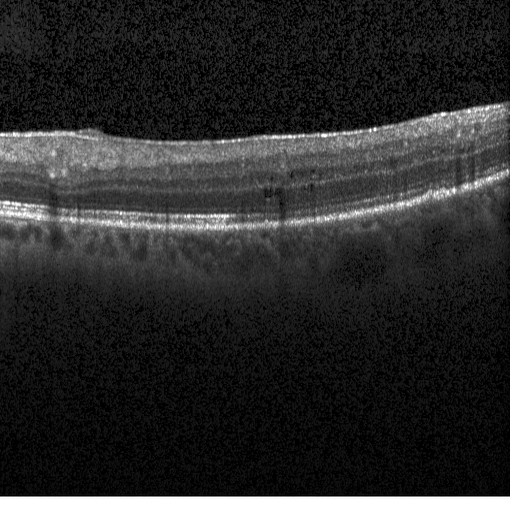

Spectral-domain optical coherence tomography · OCT B-scan — OCT finding: diabetic macular edema (DME).